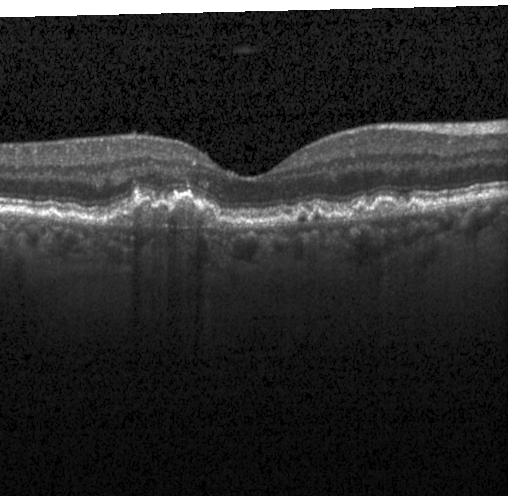
Impression: a choroidal neovascular membrane.